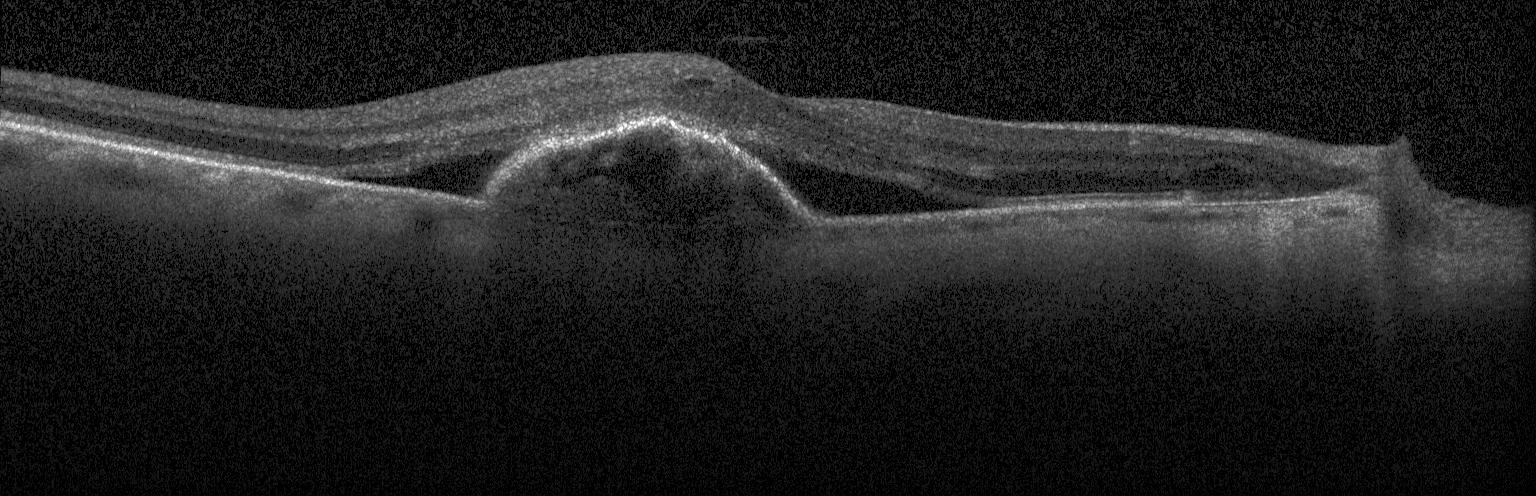

Diagnosis: a choroidal neovascular membrane.